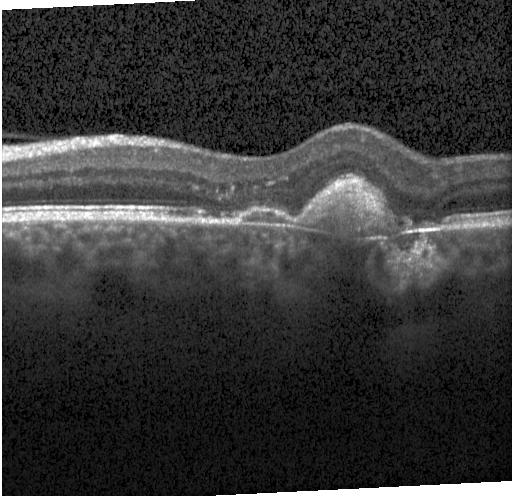
Choroidal neovascularization.